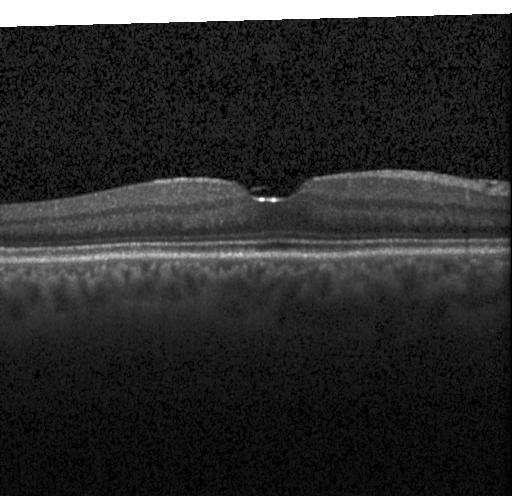 Retinal OCT B-scan, spectral-domain optical coherence tomography, horizontal scan through the fovea, Heidelberg Spectralis
Diagnosis: no evidence of choroidal neovascularization, diabetic macular edema, or drusen.